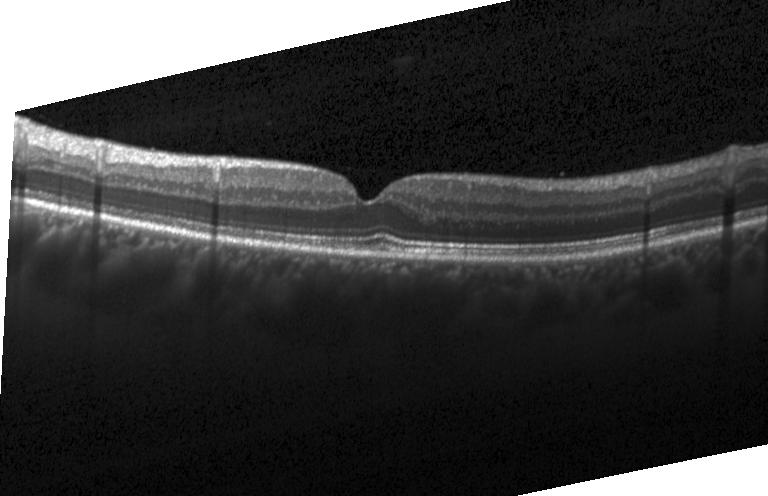

Acquired on a Heidelberg Spectralis. Optical coherence tomography B-scan. Spectral-domain optical coherence tomography — Impression: no evidence of CNV, DME, or drusen.